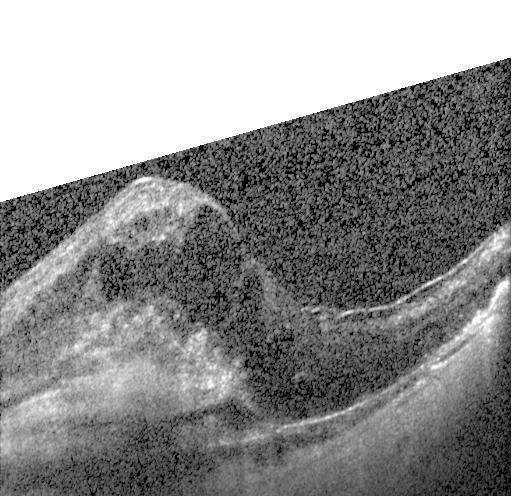 Finding: a choroidal neovascular membrane.